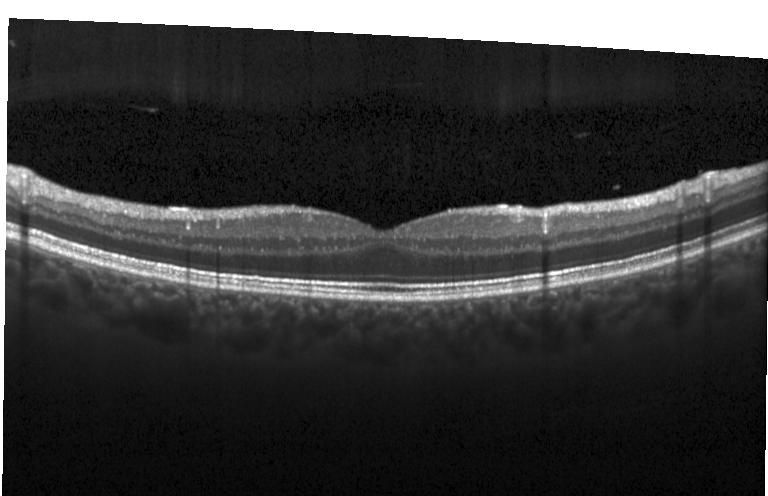

Impression: no choroidal neovascularization, diabetic macular edema, or drusen.